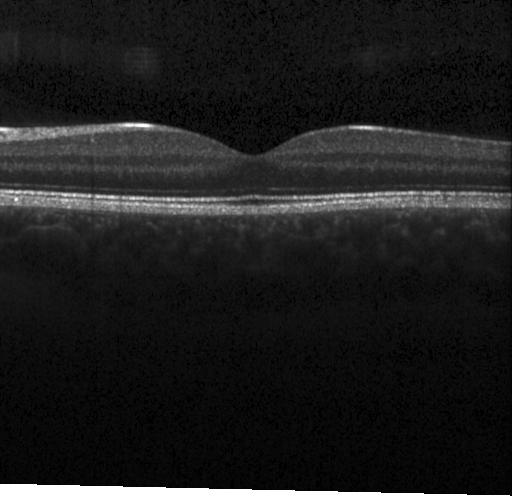 Impression: no choroidal neovascularization, diabetic macular edema, or drusen.